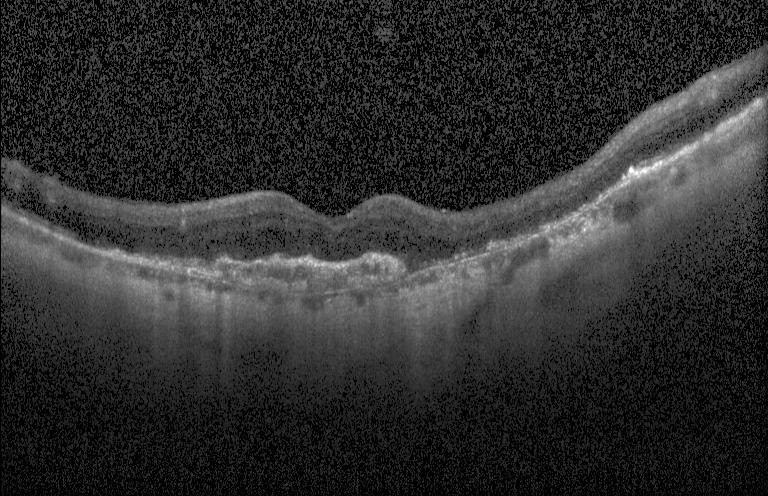 OCT line scan.
Impression: a choroidal neovascular membrane.